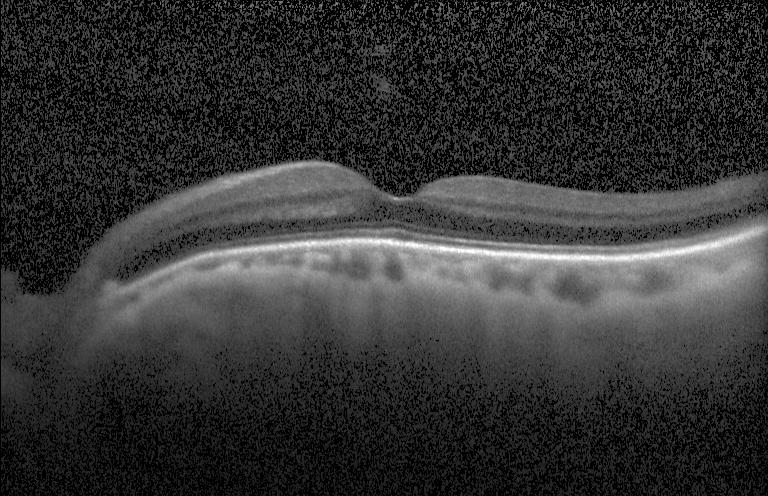
OCT line scan. Macular OCT: no choroidal neovascularization, diabetic macular edema, or drusen.